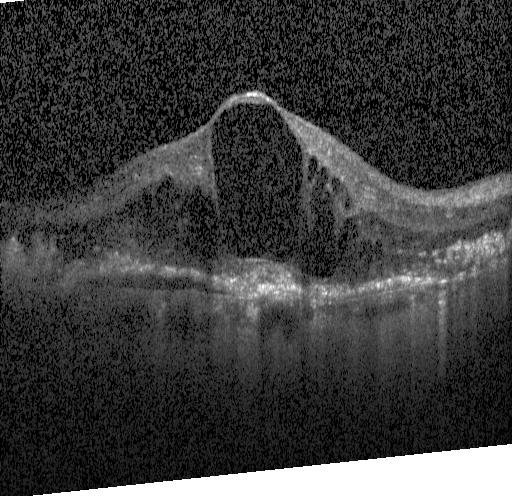

Optical coherence tomography scan
This B-scan demonstrates a choroidal neovascular membrane.